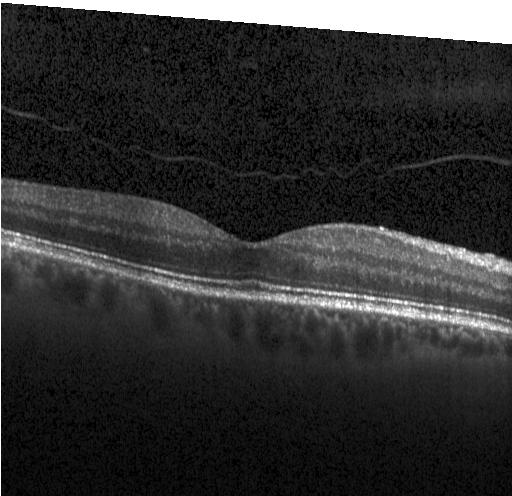

Impression: neither choroidal neovascularization, diabetic macular edema, nor drusen.